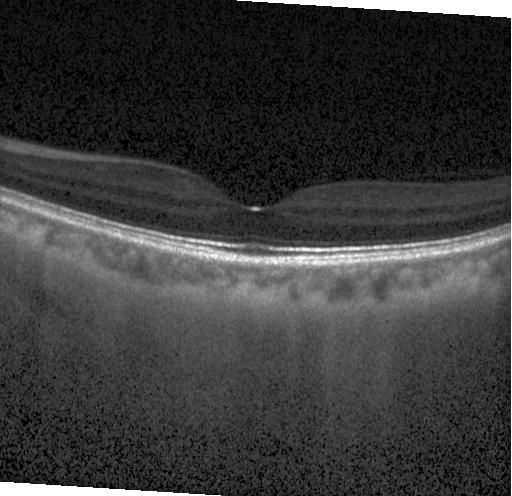 OCT B-scan. Spectral-domain OCT — No choroidal neovascularization, no diabetic macular edema, and no drusen.